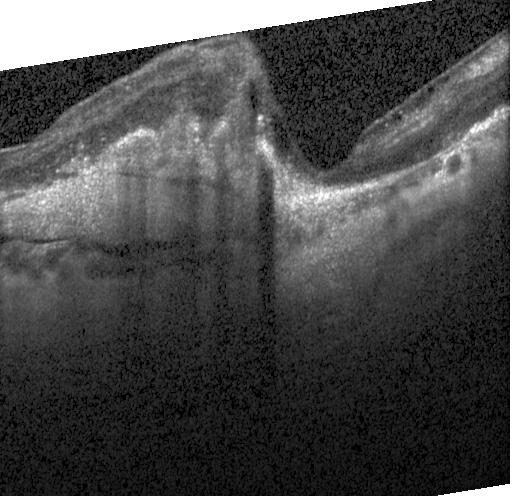 Fovea-centered · optical coherence tomography B-scan · SD-OCT · acquired on a Heidelberg Spectralis.
Impression: a choroidal neovascular membrane.